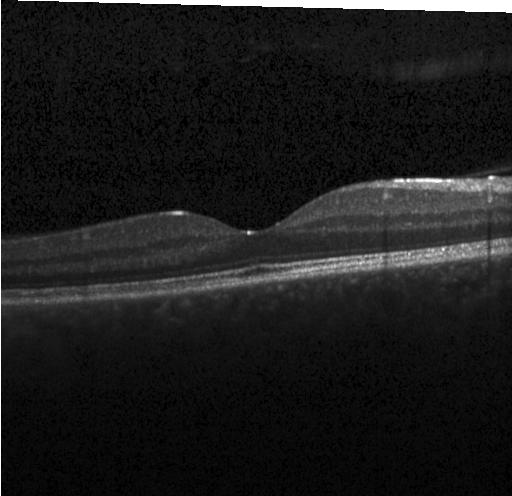
Optical coherence tomography B-scan — Assessment: neither CNV, DME, nor drusen.